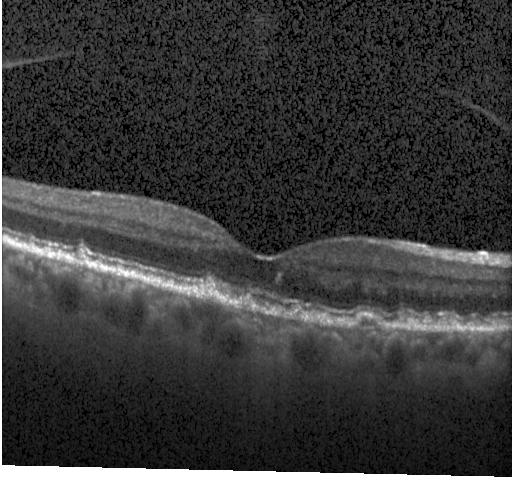
Dx: multiple drusen.